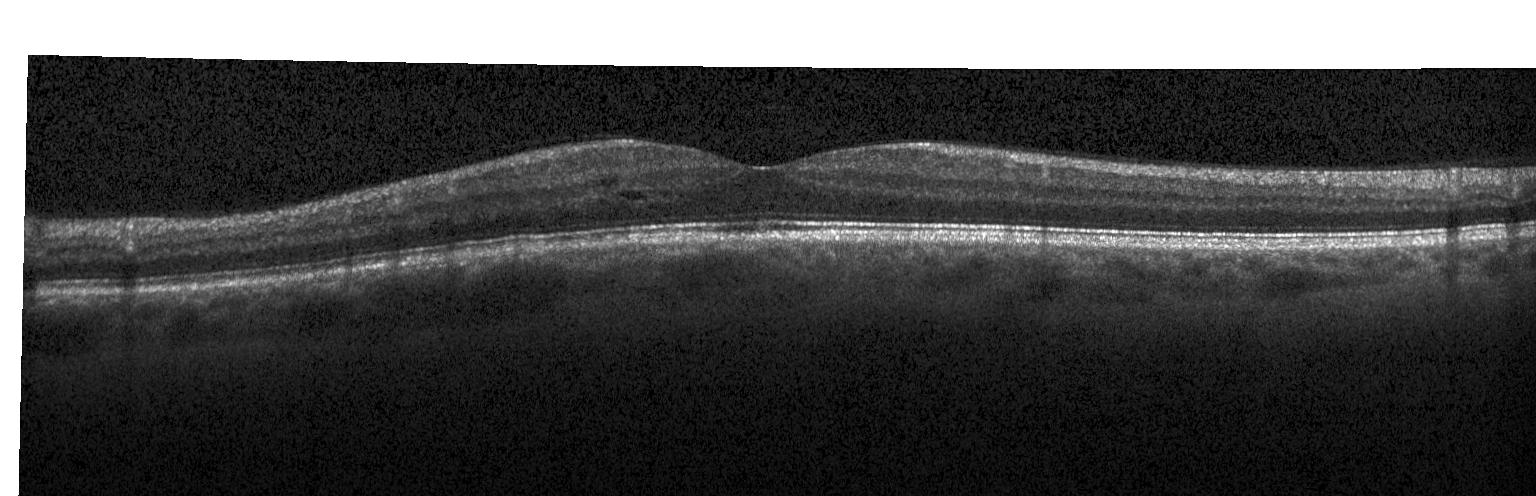
Heidelberg Spectralis OCT system. OCT line scan. SD-OCT
Macular OCT: diabetic macular edema.